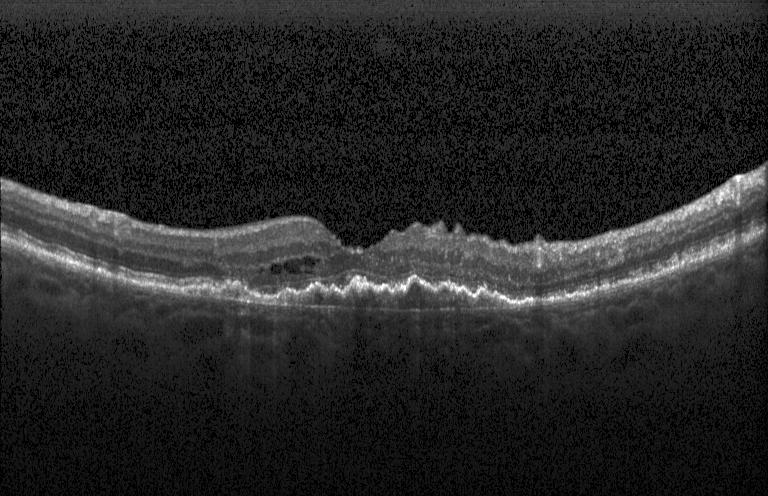
Retinal OCT B-scan; Heidelberg Spectralis
This B-scan demonstrates CNV.